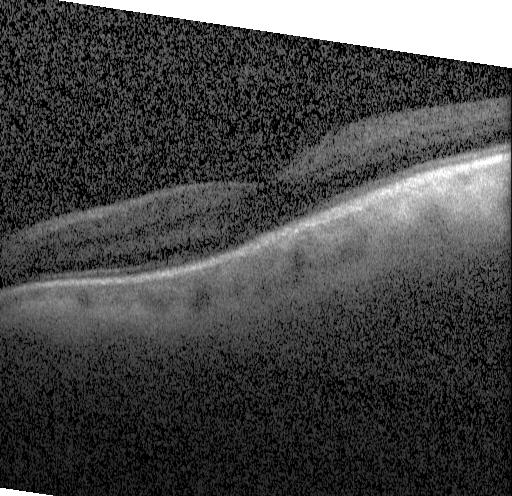
OCT scan showing neither choroidal neovascularization, diabetic macular edema, nor drusen.